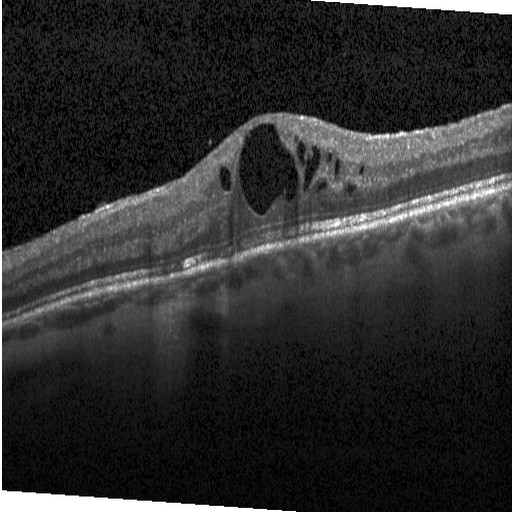
OCT scan showing DME.